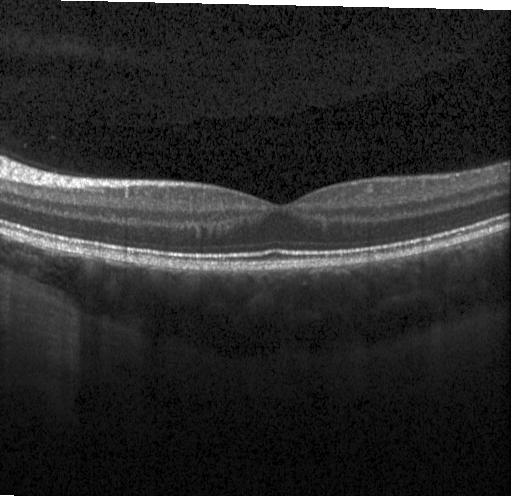

Optical coherence tomography scan
Impression: neither choroidal neovascularization, diabetic macular edema, nor drusen.